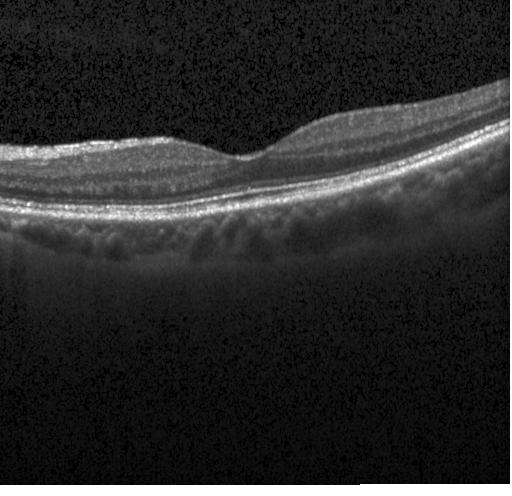 Optical coherence tomography scan, Heidelberg Spectralis. Neither CNV, DME, nor drusen.